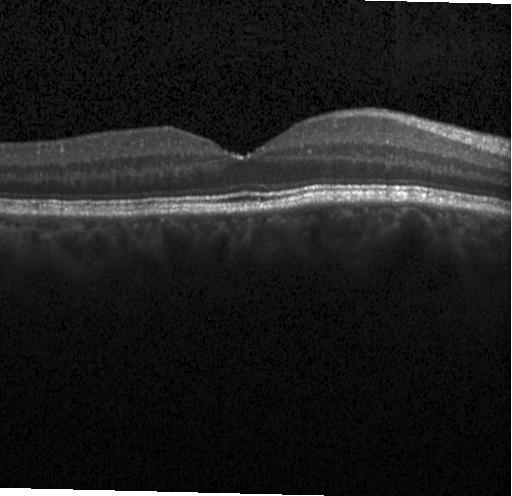
Retinal OCT cross-section showing no choroidal neovascularization, diabetic macular edema, or drusen.